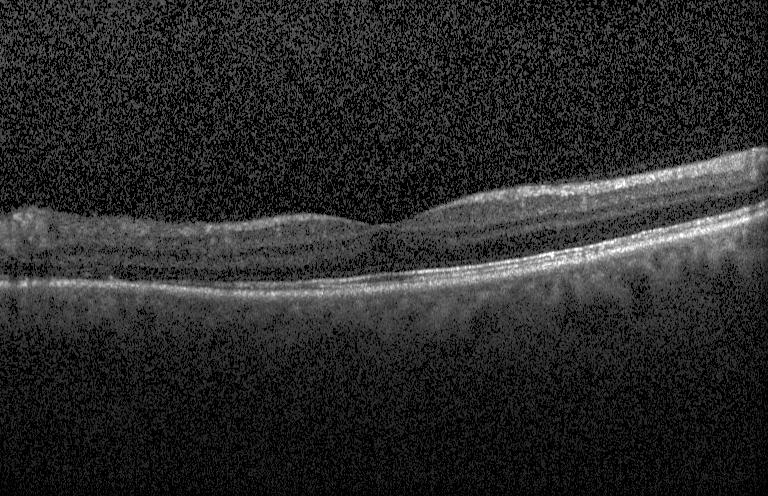

Diagnosis: no choroidal neovascularization, no diabetic macular edema, and no drusen.